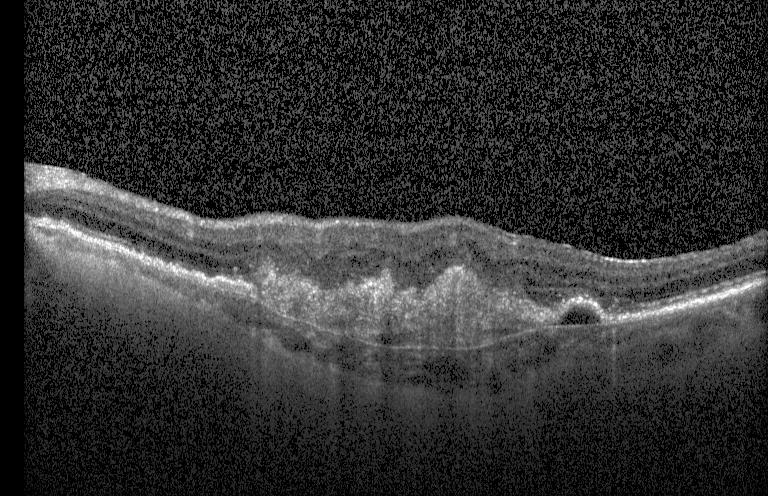 Dx: choroidal neovascularization.